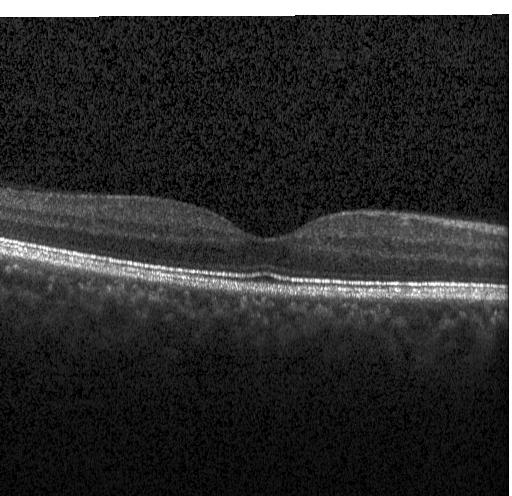

OCT line scan
This B-scan demonstrates neither choroidal neovascularization, diabetic macular edema, nor drusen.